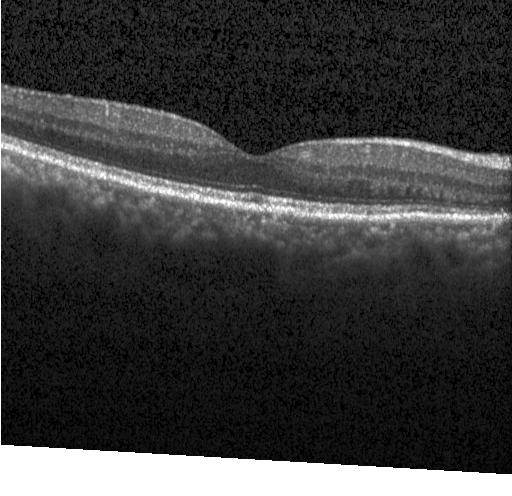 OCT B-scan. Macular scan. Acquired on a Heidelberg Spectralis. Spectral-domain OCT. Diagnosis: no choroidal neovascularization, no diabetic macular edema, and no drusen.